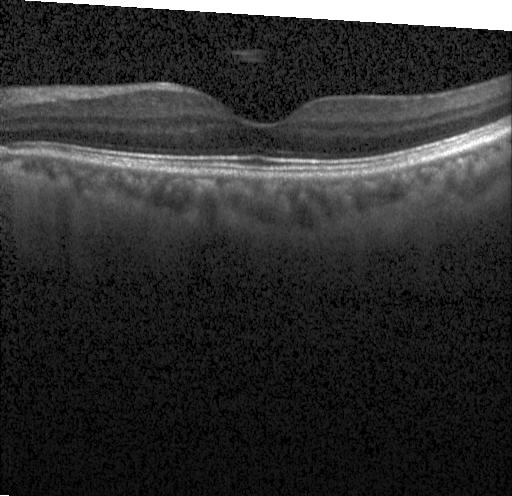

OCT B-scan. Heidelberg Spectralis. Macular scan. The scan shows no evidence of CNV, DME, or drusen.